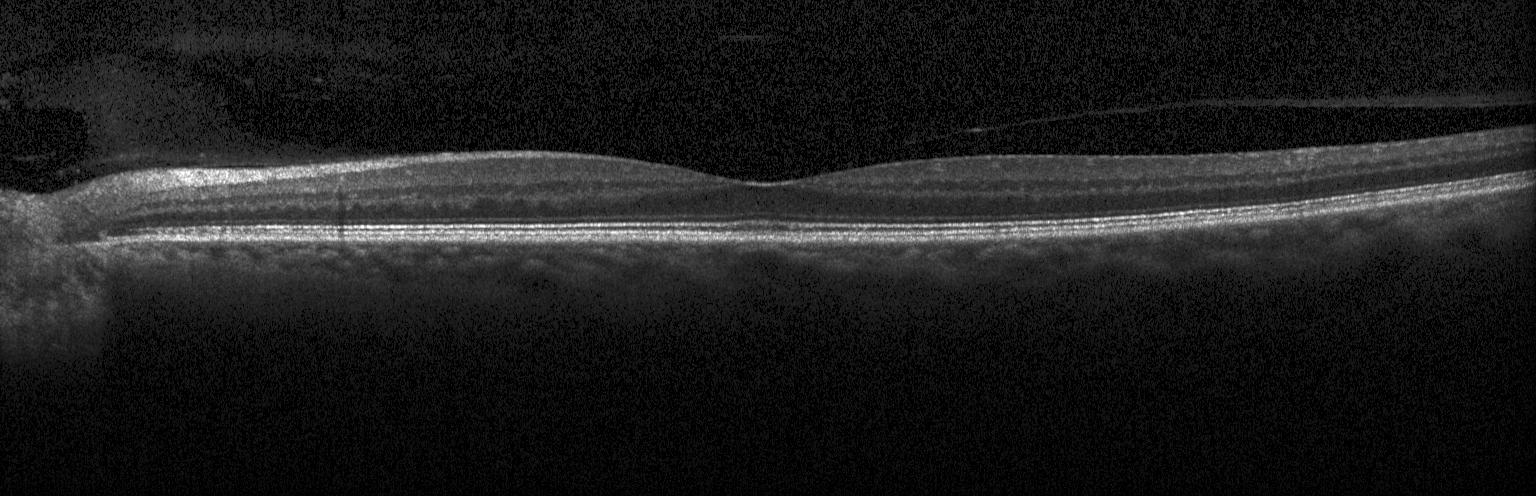
Spectral-domain OCT · optical coherence tomography B-scan · macular scan
This B-scan demonstrates no choroidal neovascularization, diabetic macular edema, or drusen.